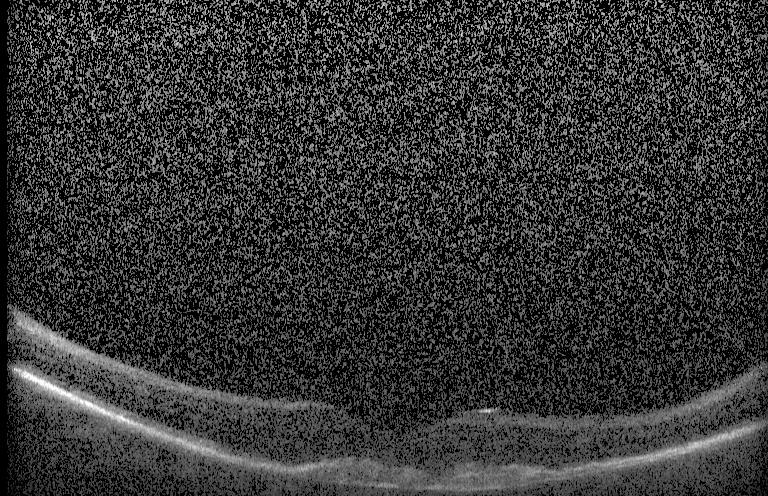
Centered on the fovea · spectral-domain optical coherence tomography · acquired on a Heidelberg Spectralis · OCT line scan.
OCT finding: choroidal neovascularization (CNV).